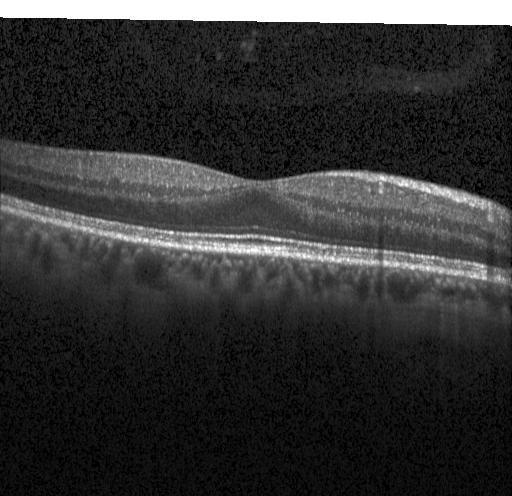

Fovea-centered. Spectral-domain OCT. Optical coherence tomography scan. Acquired on a Heidelberg Spectralis. OCT finding: no evidence of choroidal neovascularization, diabetic macular edema, or drusen.